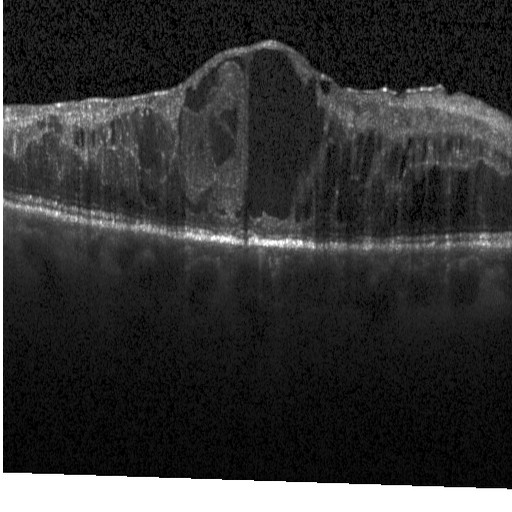
Impression: DME.